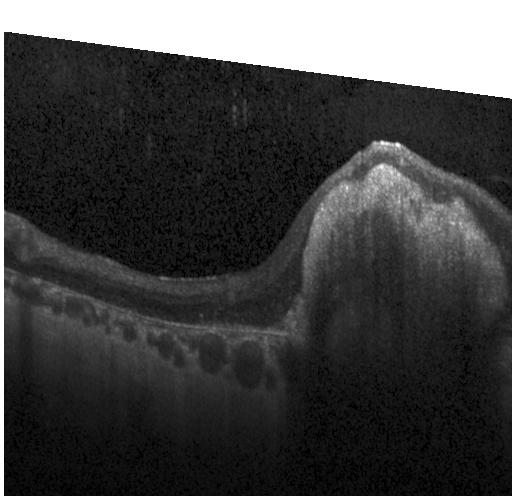
This B-scan demonstrates choroidal neovascularization.